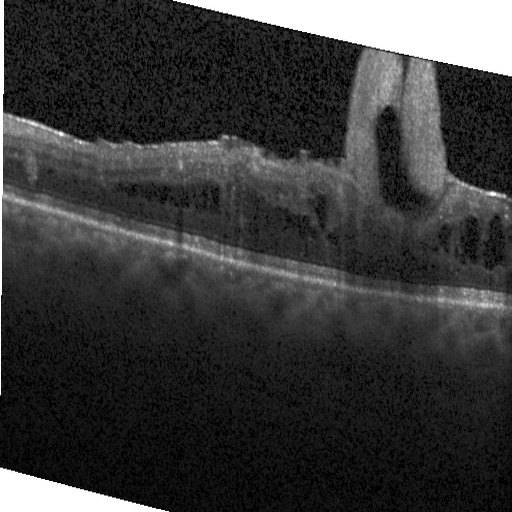
Spectral-domain OCT B-scan: diabetic macular edema.